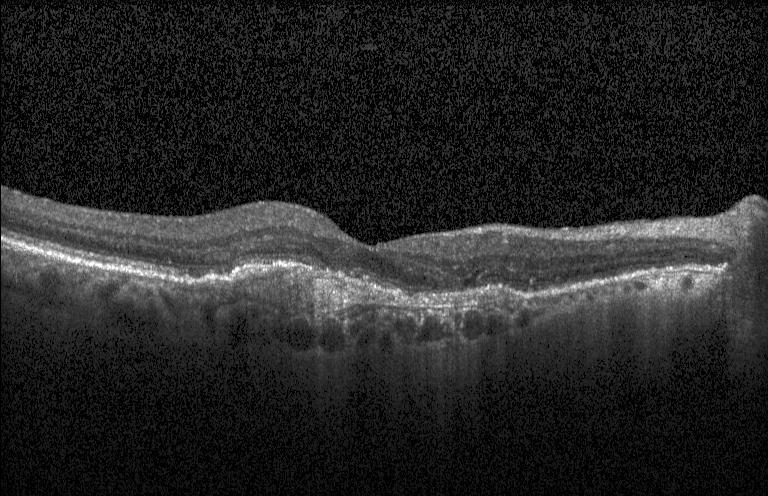
Spectral-domain OCT · retinal OCT cross-section · instrument: Heidelberg Spectralis. Macular OCT: CNV.